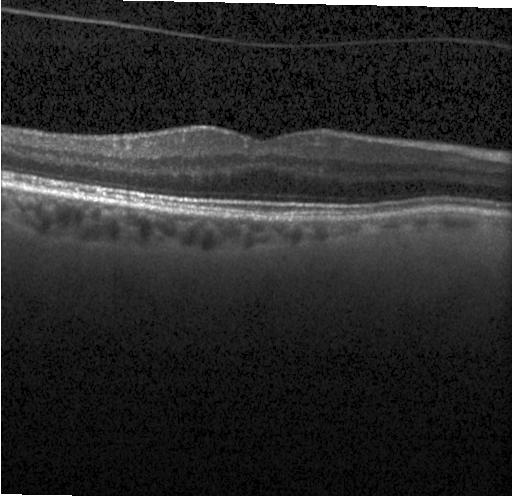
Impression: neither choroidal neovascularization, diabetic macular edema, nor drusen.